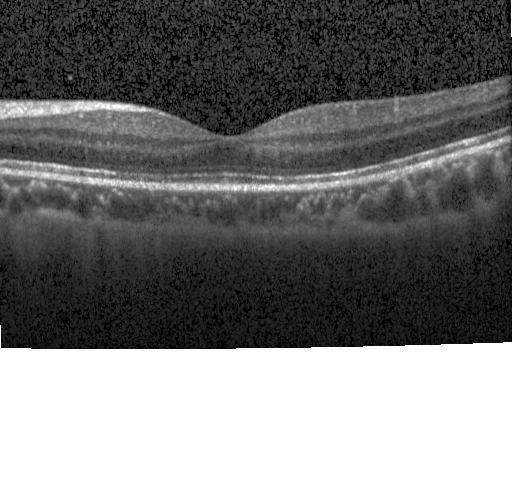 Heidelberg Spectralis OCT system, OCT line scan, centered on the fovea.
This B-scan demonstrates no CNV, DME, or drusen.